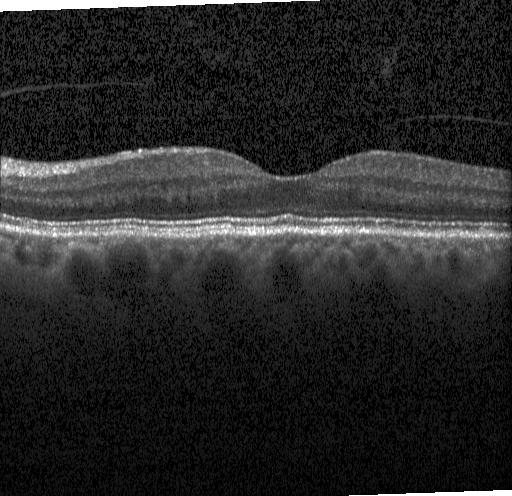 OCT line scan; acquired on a Heidelberg Spectralis; spectral-domain OCT; macular scan. OCT finding: no evidence of CNV, DME, or drusen.